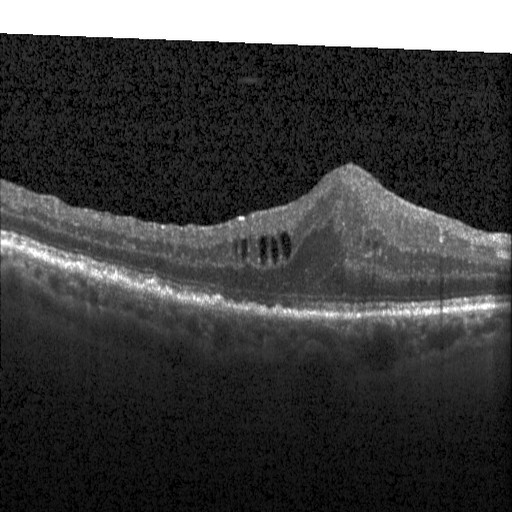 Retinal OCT cross-section; instrument: Heidelberg Spectralis; centered on the fovea. Impression: diabetic macular edema (DME).